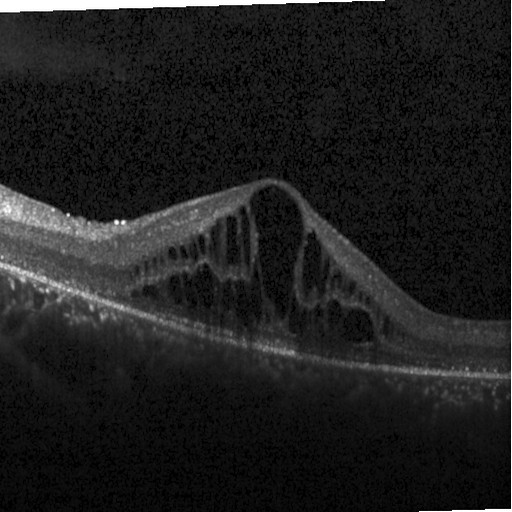 Spectral-domain OCT; horizontal scan through the fovea; Heidelberg Spectralis; optical coherence tomography B-scan
This B-scan demonstrates diabetic macular edema.